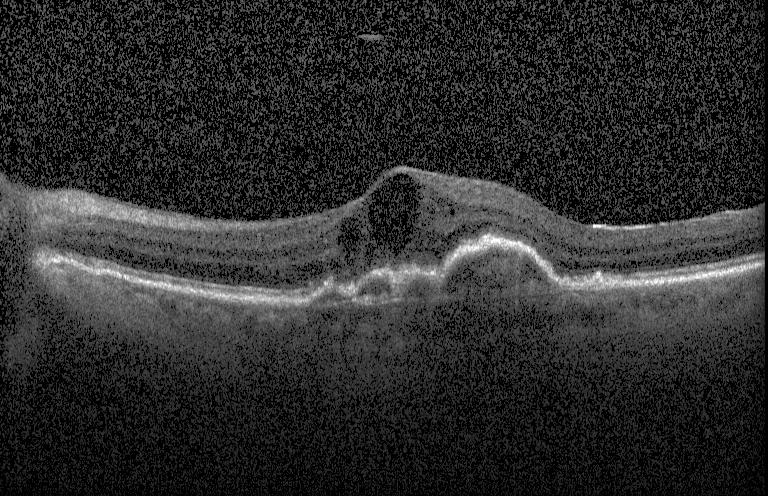
Macular OCT demonstrating CNV.